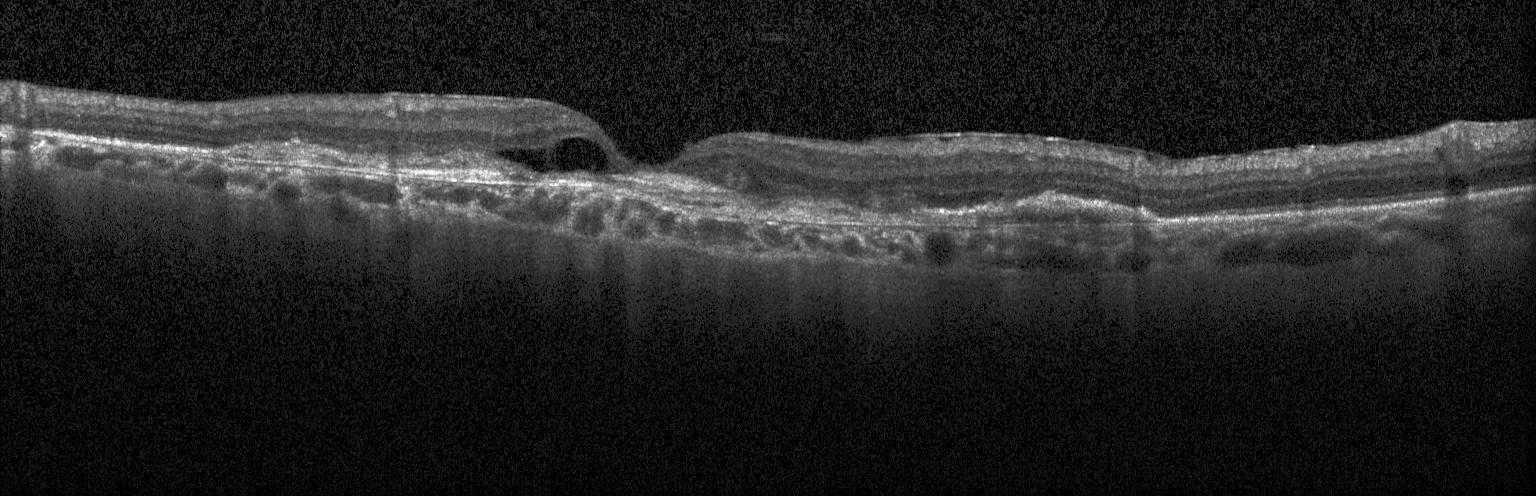 OCT B-scan showing CNV.